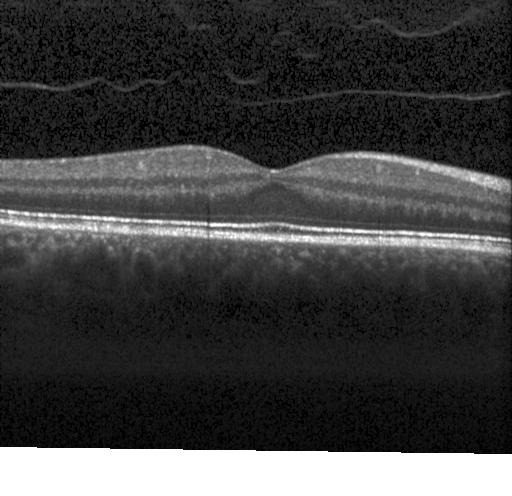

Retinal OCT cross-section, centered on the fovea, acquired on a Heidelberg Spectralis, spectral-domain OCT.
Diagnosis: no choroidal neovascularization, no diabetic macular edema, and no drusen.